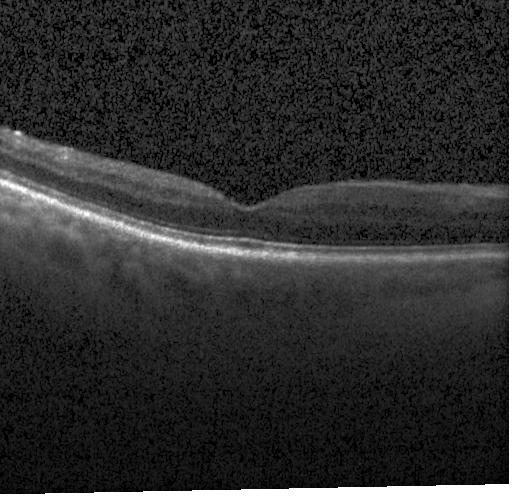
Retinal OCT B-scan — The scan shows neither choroidal neovascularization, diabetic macular edema, nor drusen.